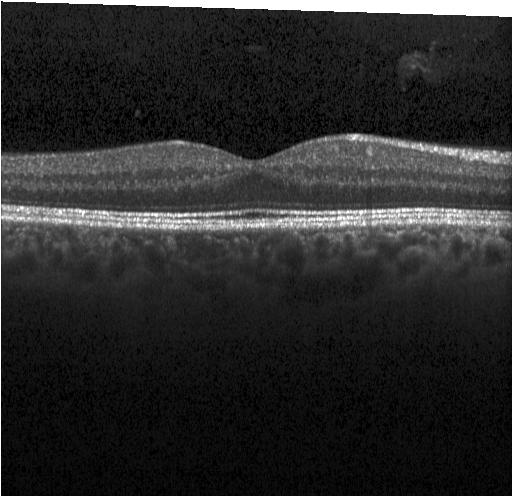
Heidelberg Spectralis; spectral-domain OCT; OCT B-scan.
Diagnosis: no evidence of choroidal neovascularization, diabetic macular edema, or drusen.